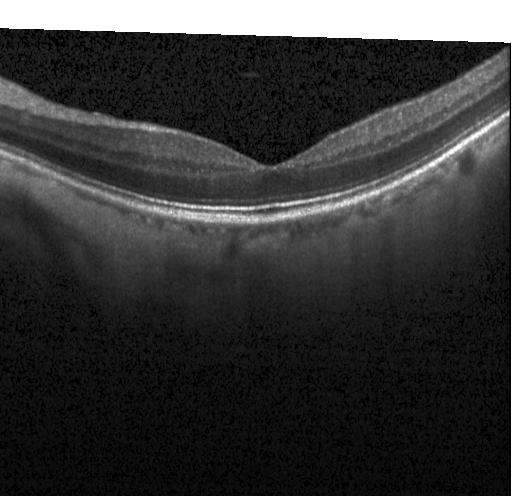 Through the macula. Heidelberg Spectralis. Spectral-domain OCT. Retinal OCT B-scan
Macular OCT: no choroidal neovascularization, diabetic macular edema, or drusen.